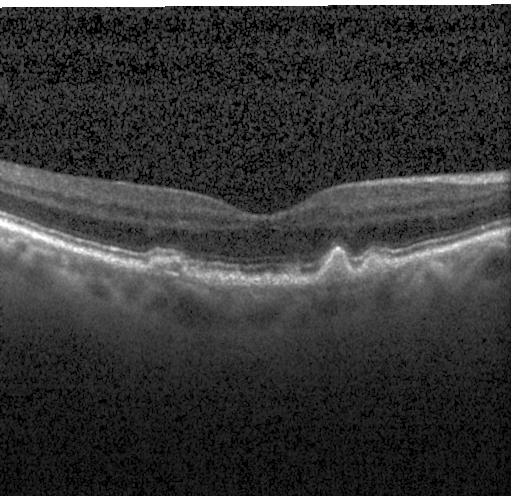

Retinal OCT B-scan; fovea-centered
OCT finding: multiple drusen.